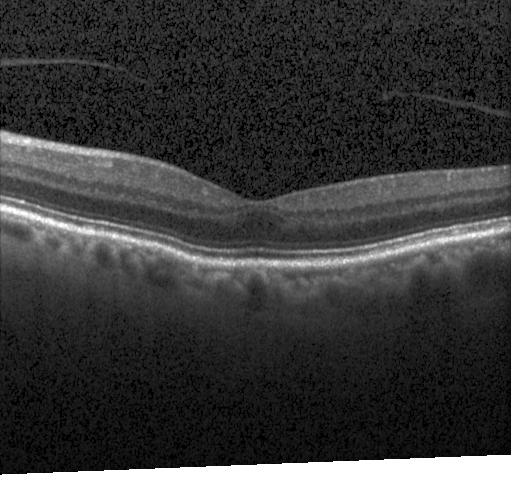
Through the macula, OCT B-scan, spectral-domain OCT — Finding: neither choroidal neovascularization, diabetic macular edema, nor drusen.